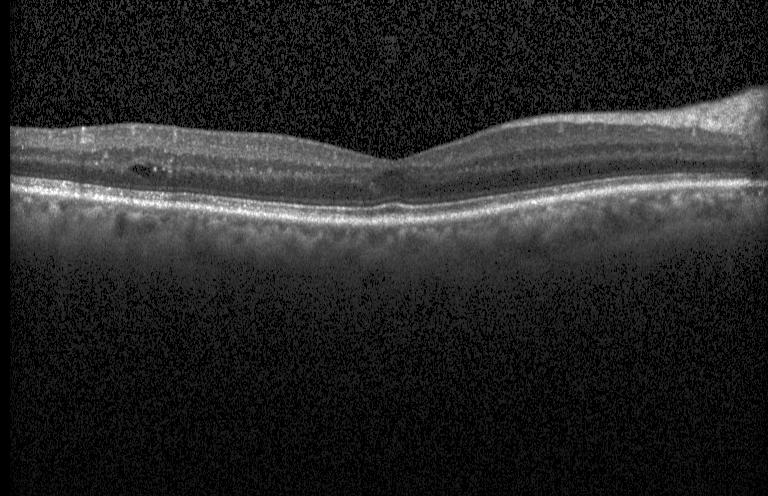

SD-OCT; instrument: Heidelberg Spectralis; optical coherence tomography scan; fovea-centered
Diagnosis: diabetic macular edema.